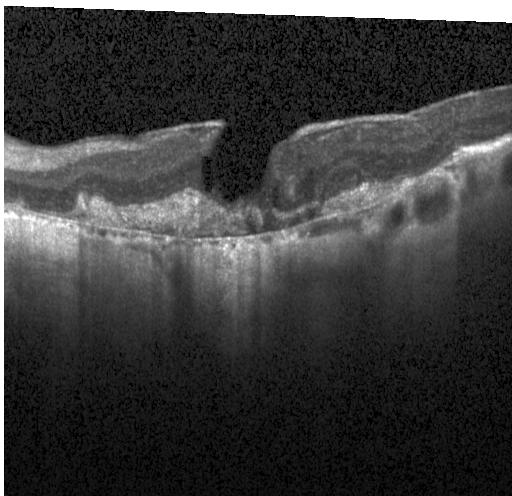
Diagnosis: a choroidal neovascular membrane.